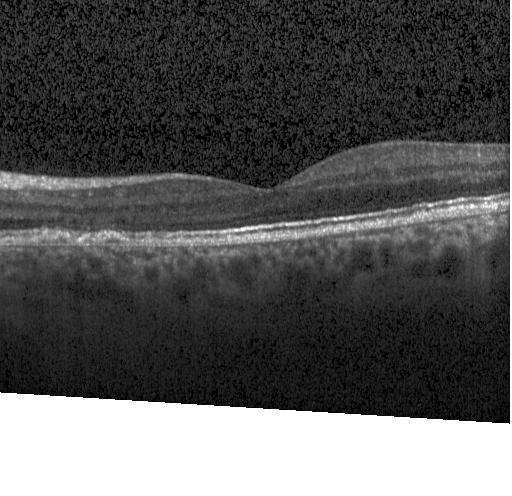 Instrument: Heidelberg Spectralis. Spectral-domain OCT. OCT B-scan
Diagnosis: CNV.